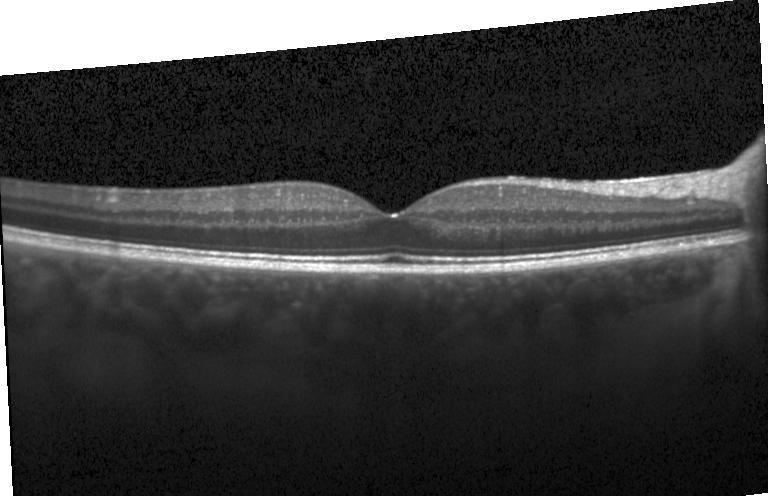 Finding: neither choroidal neovascularization, diabetic macular edema, nor drusen.